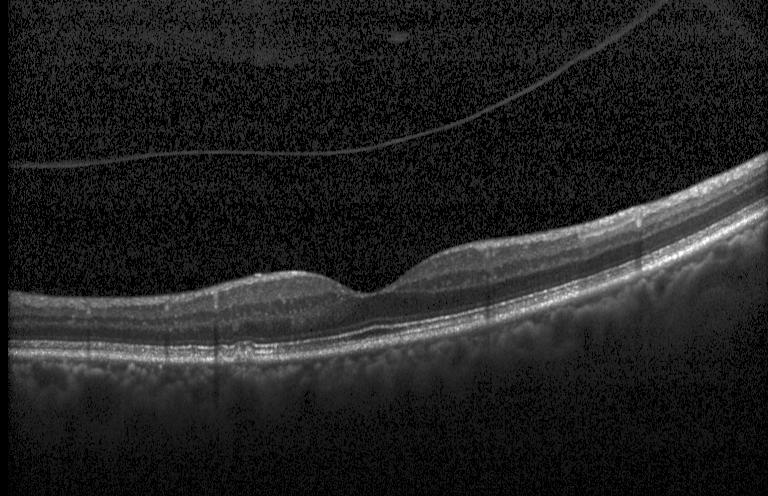 Horizontal scan through the fovea · retinal OCT B-scan · SD-OCT
Multiple drusen.